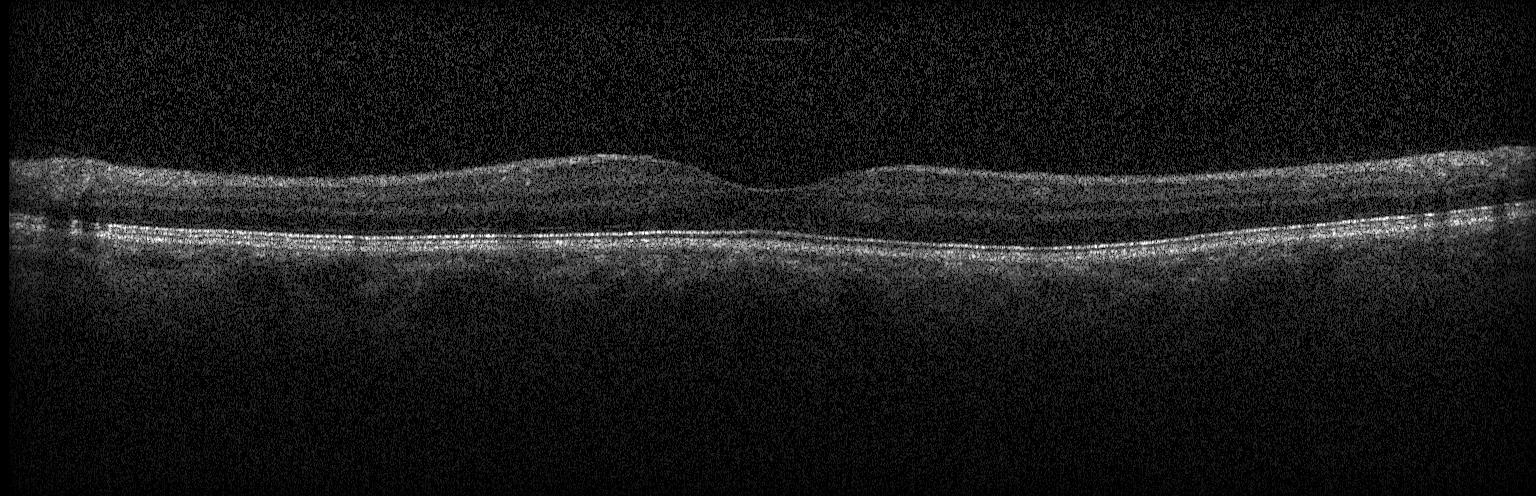
SD-OCT · optical coherence tomography B-scan
Impression: no evidence of choroidal neovascularization, diabetic macular edema, or drusen.